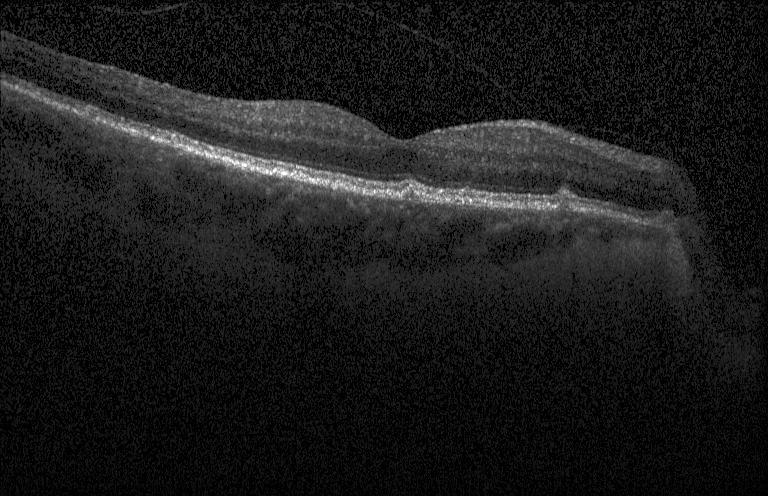 OCT B-scan · Heidelberg Spectralis · spectral-domain optical coherence tomography.
Dx: multiple drusen.